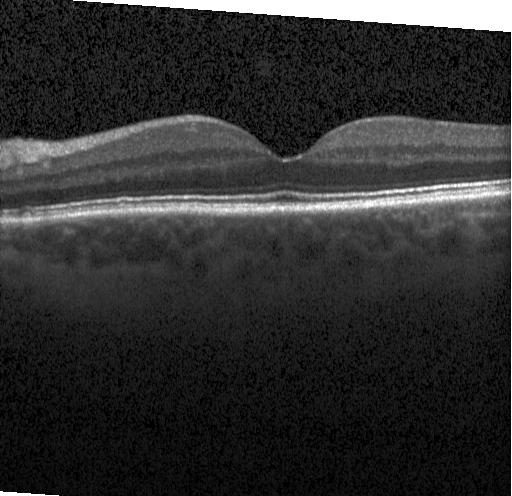 Dx: neither choroidal neovascularization, diabetic macular edema, nor drusen.